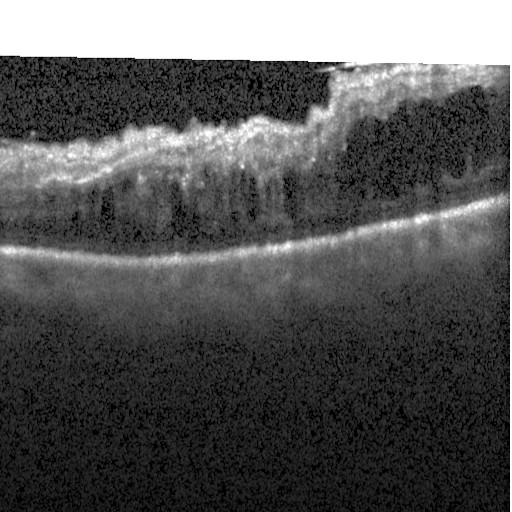 Finding: diabetic macular edema.